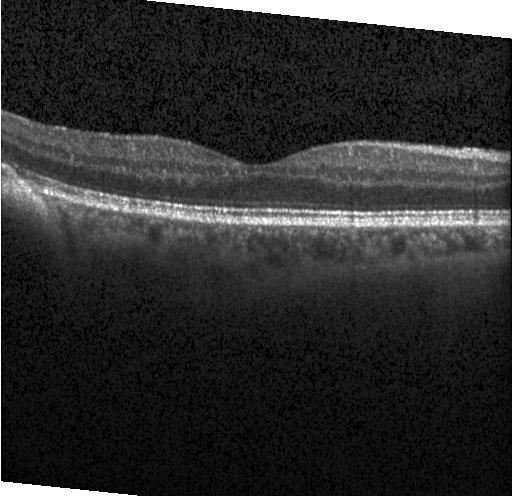
The scan shows neither choroidal neovascularization, diabetic macular edema, nor drusen.